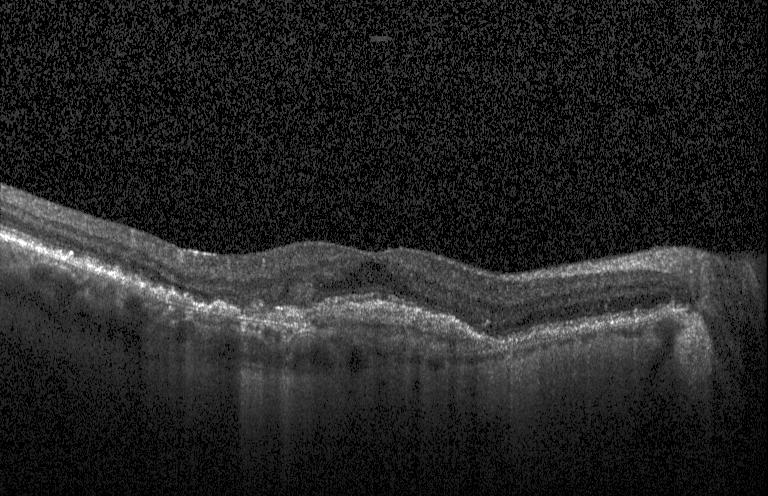

Retinal OCT B-scan. Assessment: CNV.